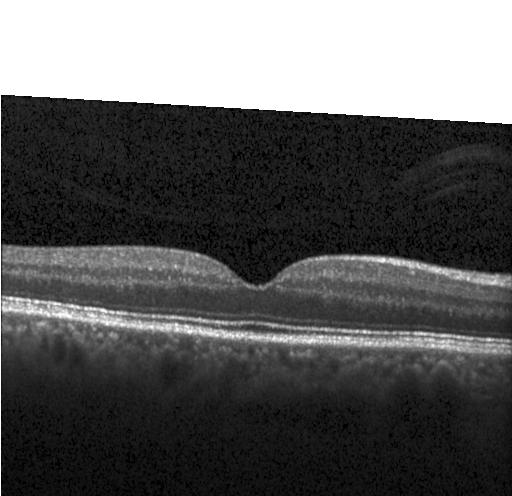

This B-scan demonstrates neither choroidal neovascularization, diabetic macular edema, nor drusen.